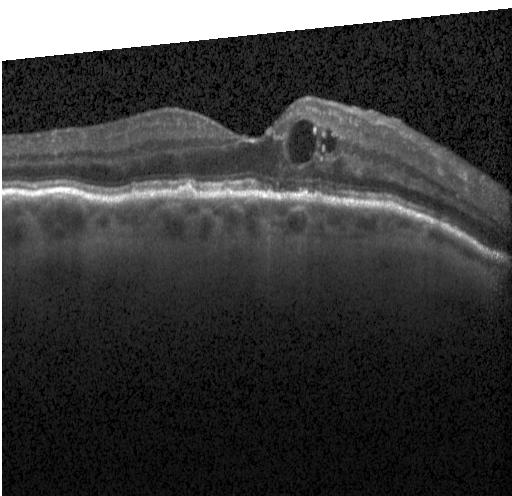
Finding: a choroidal neovascular membrane.